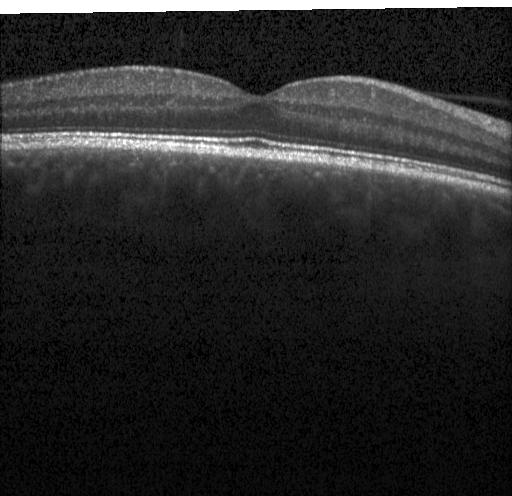 Optical coherence tomography scan, Heidelberg Spectralis, through the macula, spectral-domain OCT
Diagnosis: no evidence of CNV, DME, or drusen.